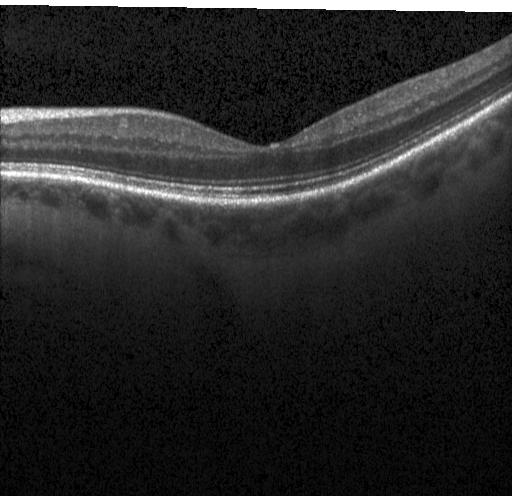

OCT B-scan showing no CNV, DME, or drusen.